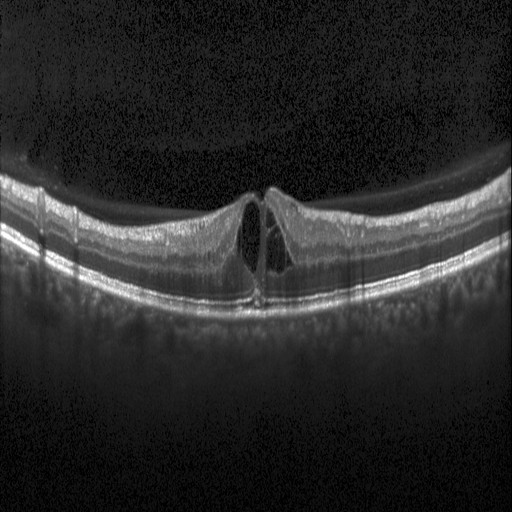
Optical coherence tomography scan, through the macula.
Diagnosis: diabetic macular edema.